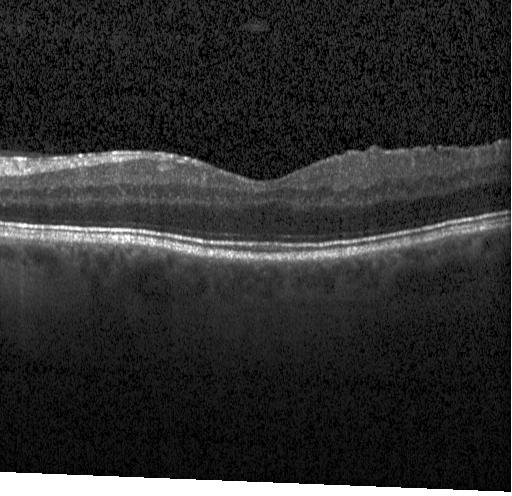

The scan shows no choroidal neovascularization, no diabetic macular edema, and no drusen.